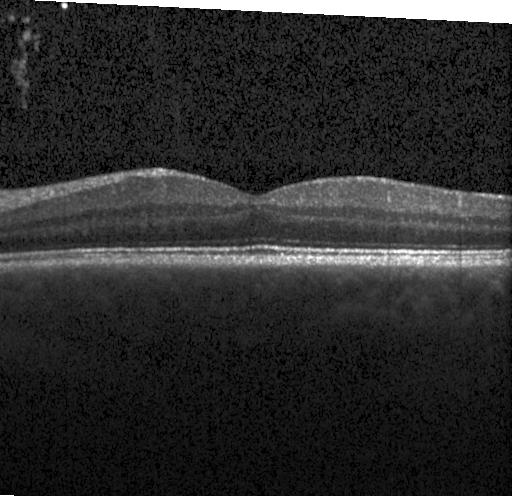
Spectral-domain OCT · Heidelberg Spectralis OCT system · retinal OCT B-scan. This B-scan demonstrates no choroidal neovascularization, diabetic macular edema, or drusen.